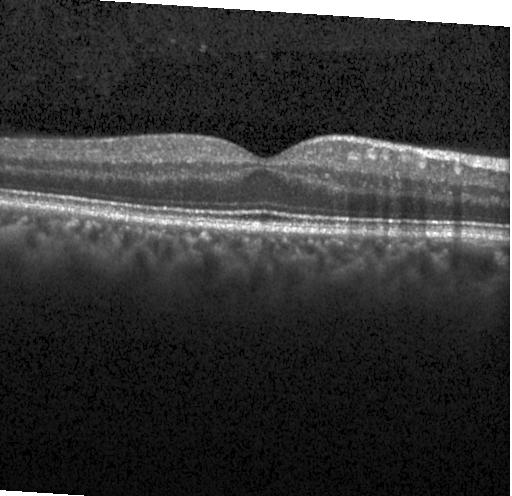

Retinal OCT cross-section.
Dx: neither choroidal neovascularization, diabetic macular edema, nor drusen.